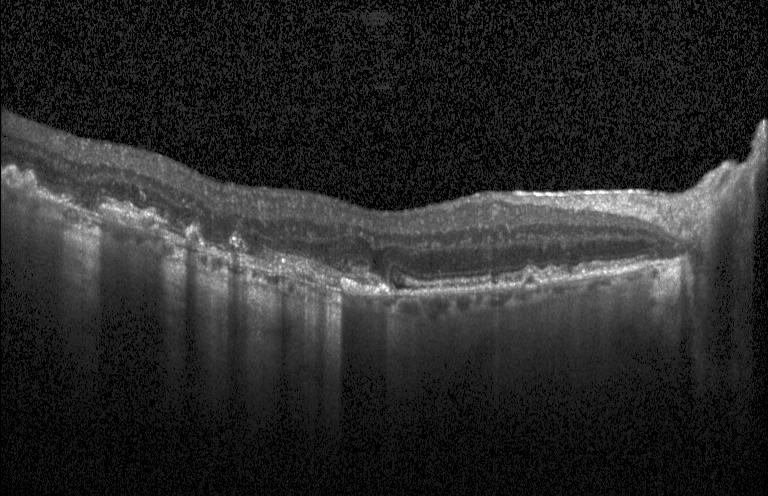 Finding: a choroidal neovascular membrane.